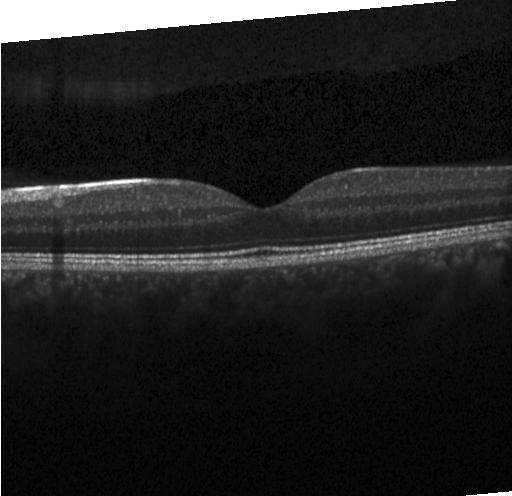
Macular scan. Retinal OCT cross-section.
Dx: no CNV, DME, or drusen.